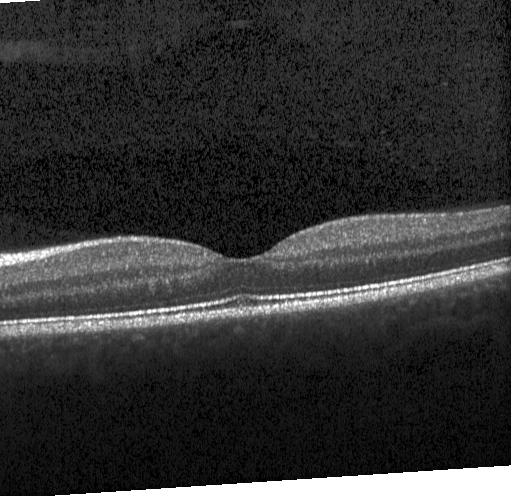 Optical coherence tomography B-scan; spectral-domain OCT
Diagnosis: no evidence of choroidal neovascularization, diabetic macular edema, or drusen.